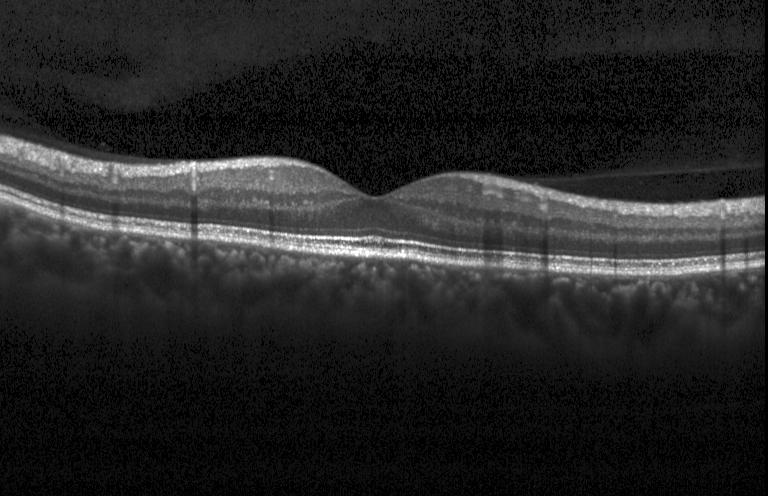 Macular OCT demonstrating neither choroidal neovascularization, diabetic macular edema, nor drusen.